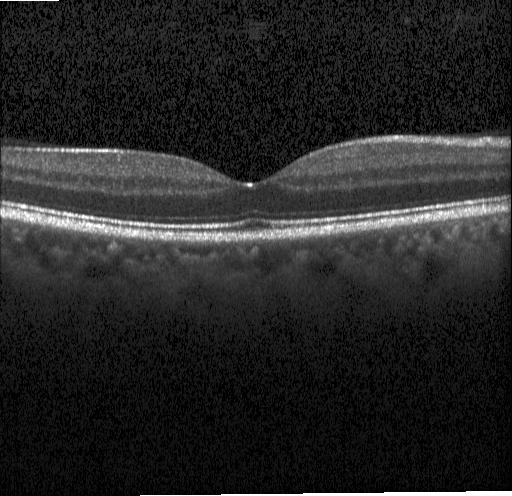 Heidelberg Spectralis OCT system, retinal OCT B-scan, SD-OCT, horizontal scan through the fovea. Impression: no evidence of choroidal neovascularization, diabetic macular edema, or drusen.